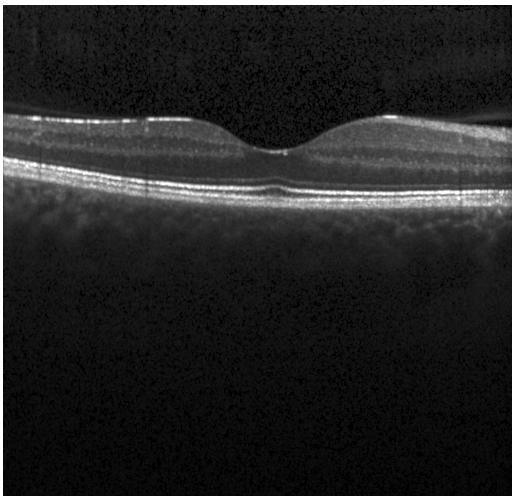

OCT B-scan; Heidelberg Spectralis
OCT finding: neither choroidal neovascularization, diabetic macular edema, nor drusen.